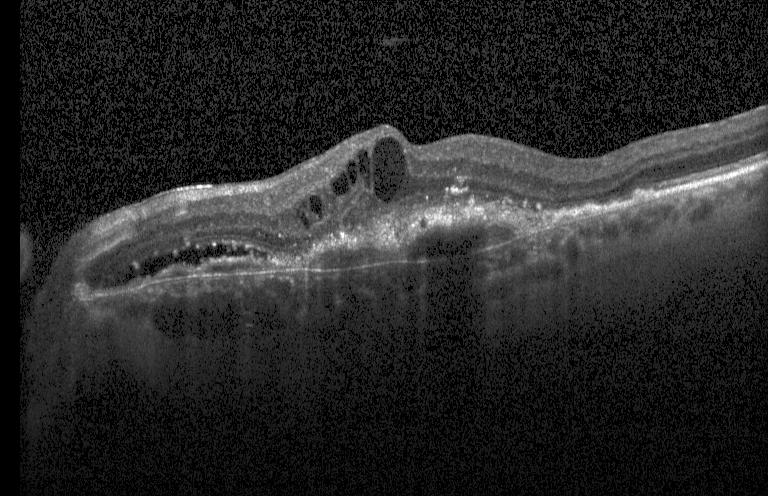 Spectral-domain optical coherence tomography. Optical coherence tomography B-scan — Impression: a choroidal neovascular membrane.